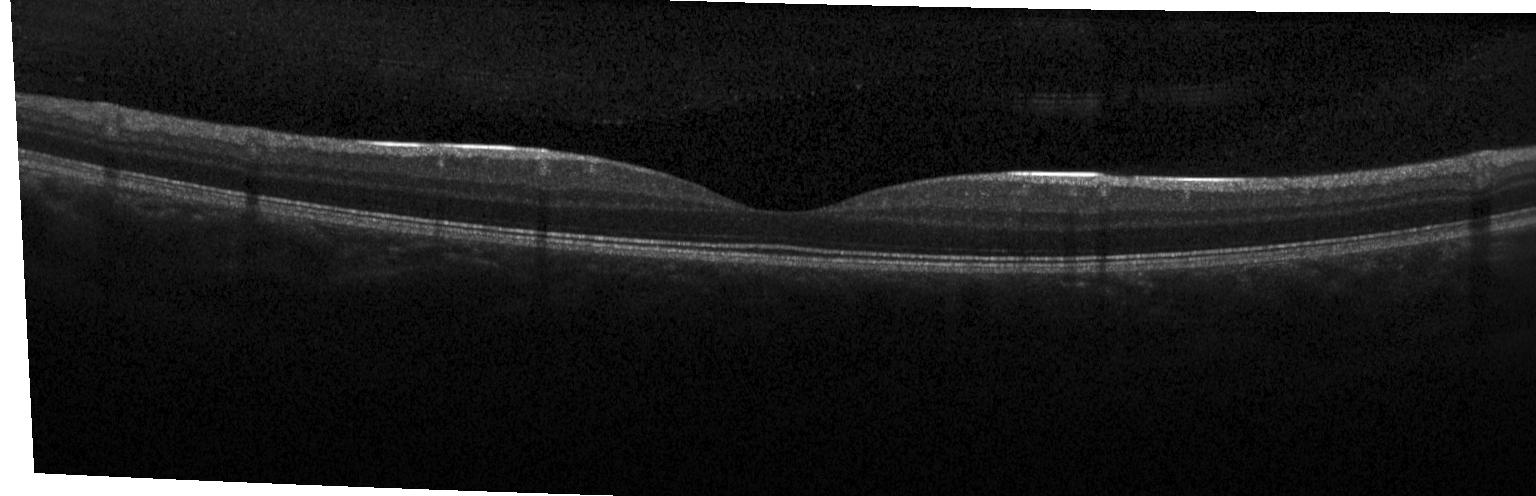 Optical coherence tomography scan
Finding: no evidence of CNV, DME, or drusen.